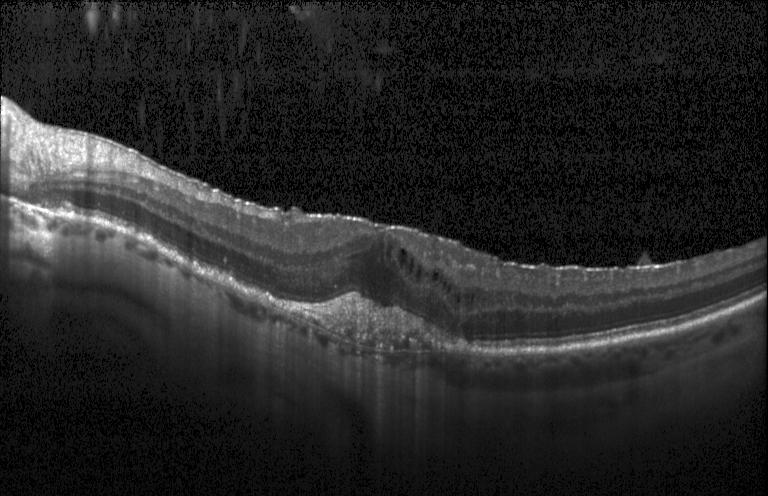
OCT B-scan — Impression: CNV.